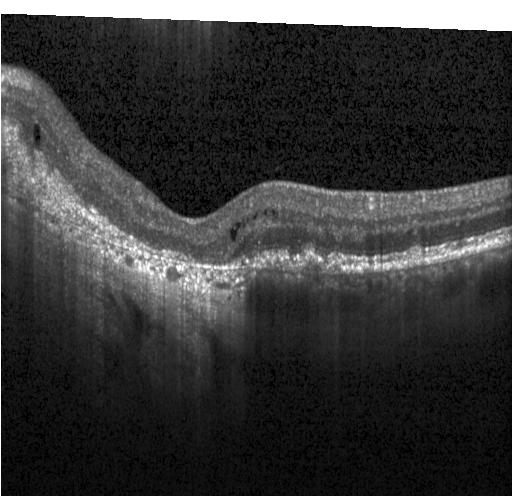
OCT finding: choroidal neovascularization (CNV).